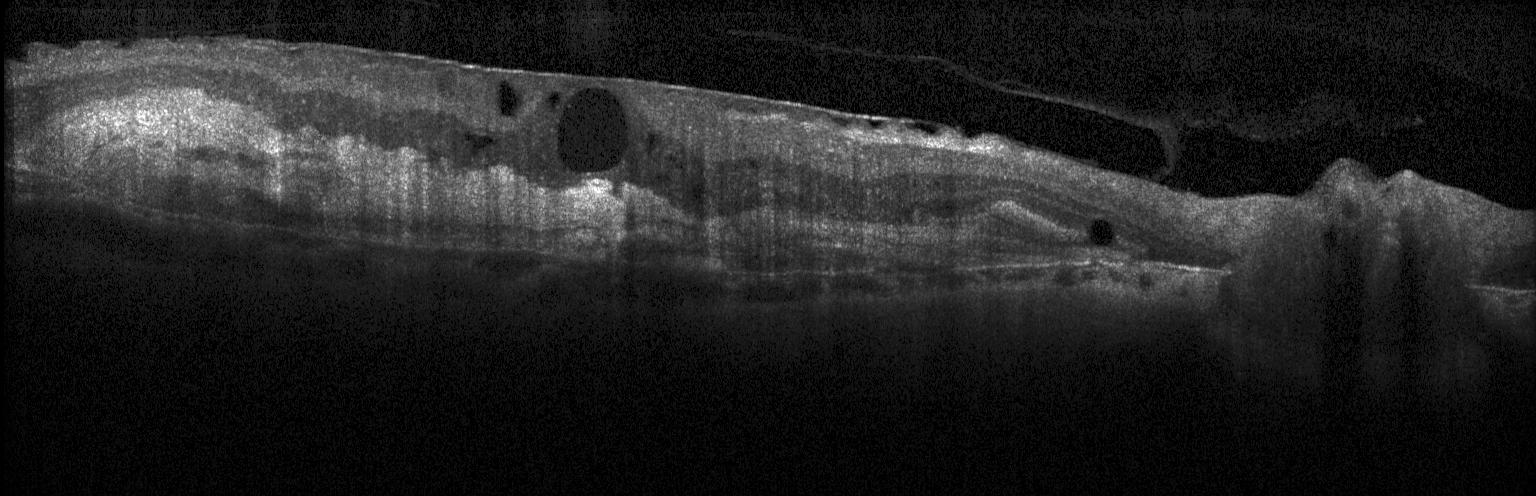
Optical coherence tomography B-scan, acquired on a Heidelberg Spectralis. Diagnosis: choroidal neovascularization.